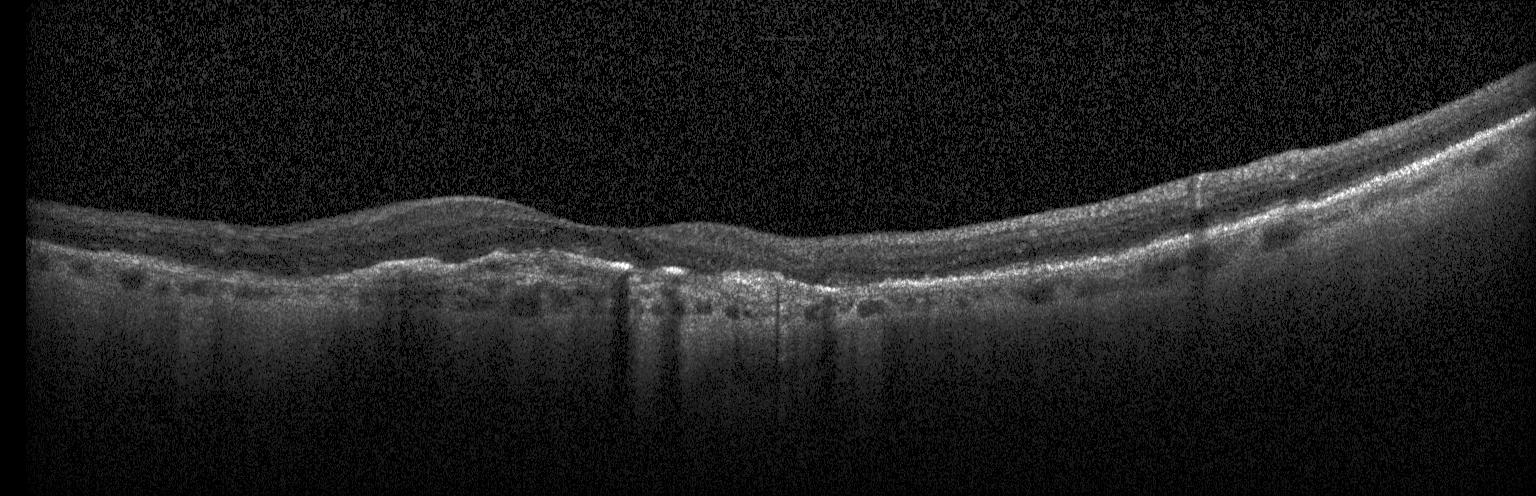
Spectral-domain OCT; centered on the fovea; retinal OCT B-scan; acquired on a Heidelberg Spectralis.
Finding: choroidal neovascularization.